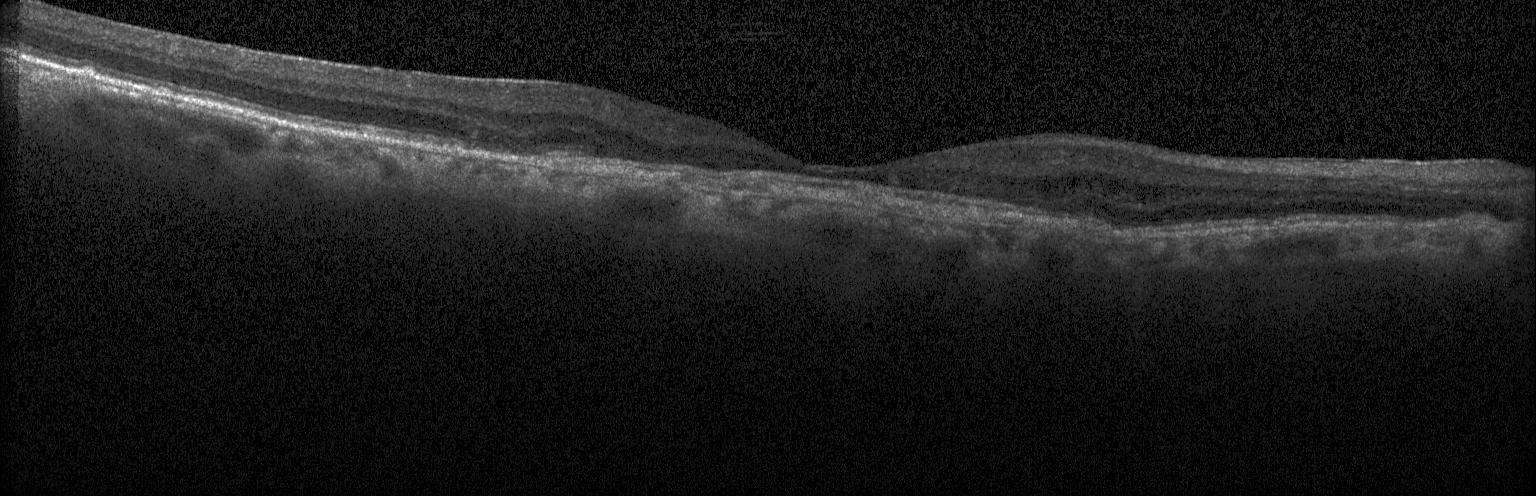
OCT finding: a choroidal neovascular membrane.